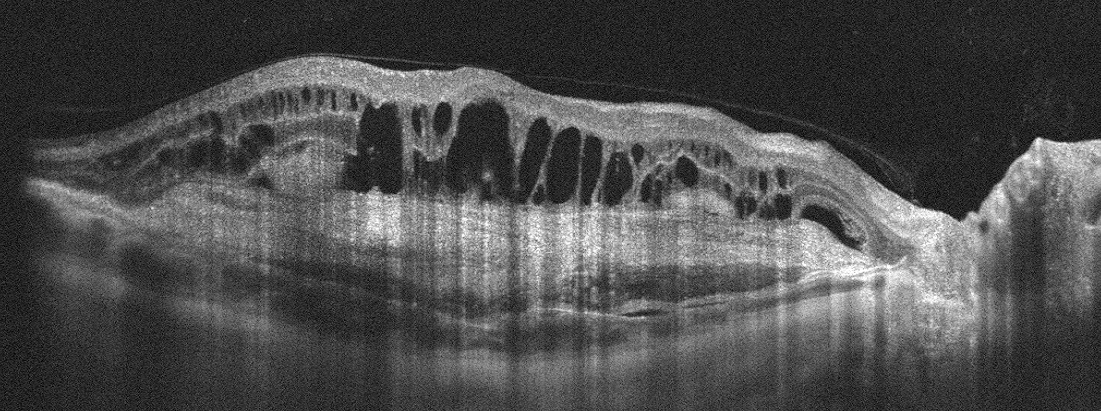 Diagnosis: age-related macular degeneration.